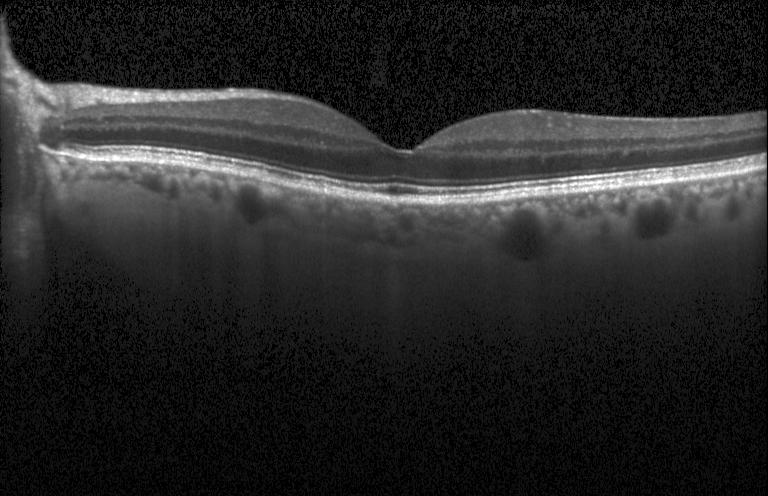 SD-OCT; through the macula; instrument: Heidelberg Spectralis; optical coherence tomography scan. Finding: no choroidal neovascularization, no diabetic macular edema, and no drusen.